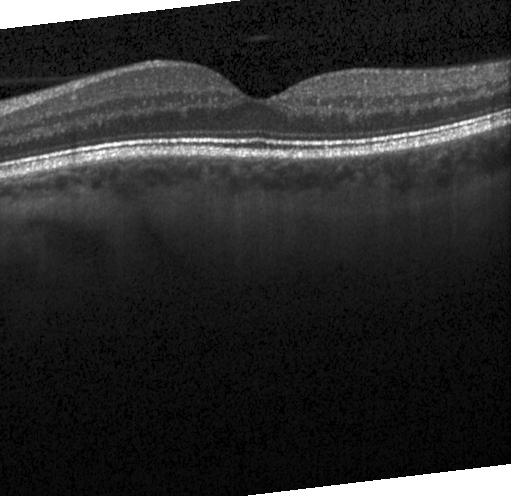

Retinal OCT B-scan, Heidelberg Spectralis OCT system
Assessment: no CNV, no DME, and no drusen.